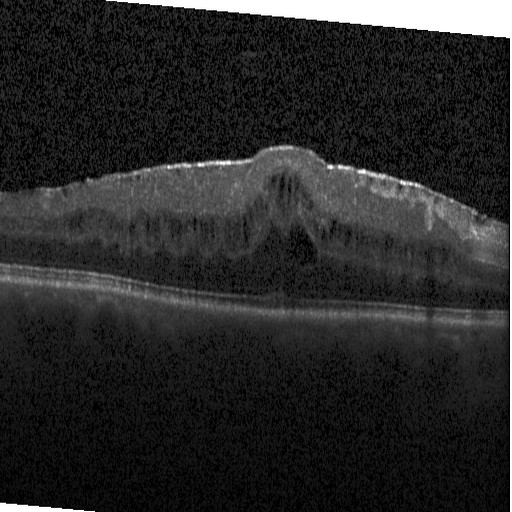

Spectral-domain optical coherence tomography, Heidelberg Spectralis, optical coherence tomography scan. Impression: DME.